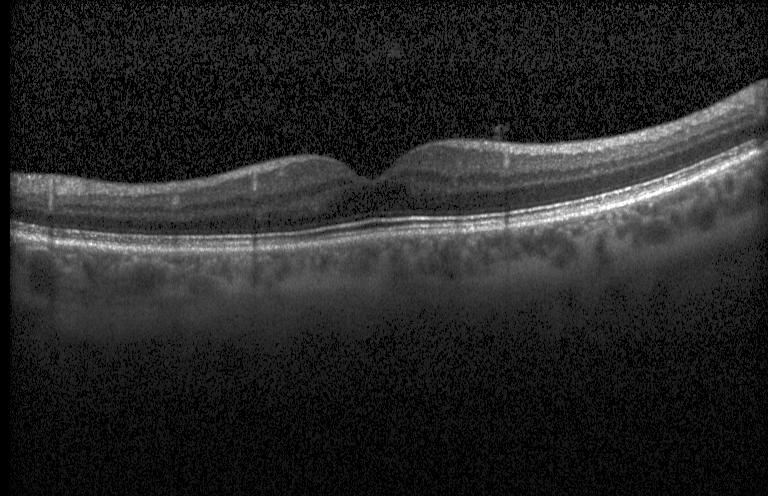

OCT finding: no choroidal neovascularization, diabetic macular edema, or drusen.